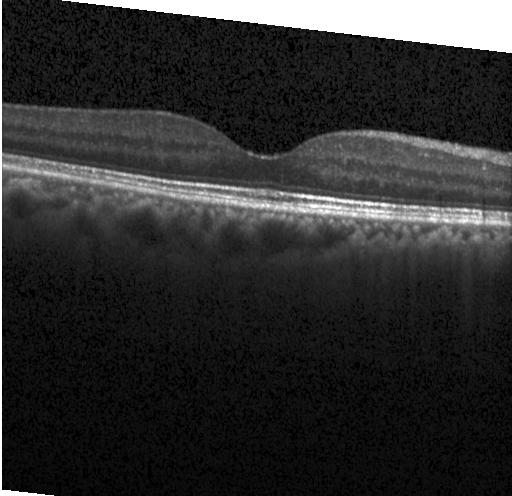 OCT B-scan.
No evidence of CNV, DME, or drusen.